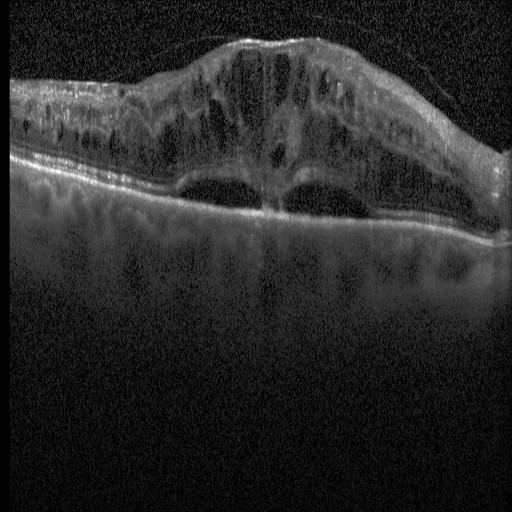

Retinal OCT B-scan — Diagnosis: diabetic macular edema.